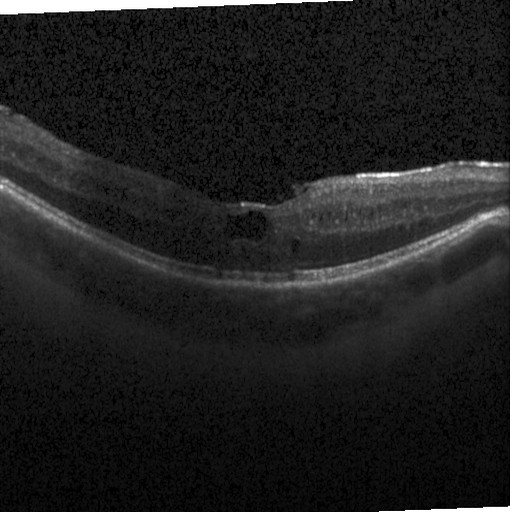
Spectral-domain OCT; horizontal scan through the fovea; retinal OCT cross-section; instrument: Heidelberg Spectralis — Impression: diabetic macular edema.